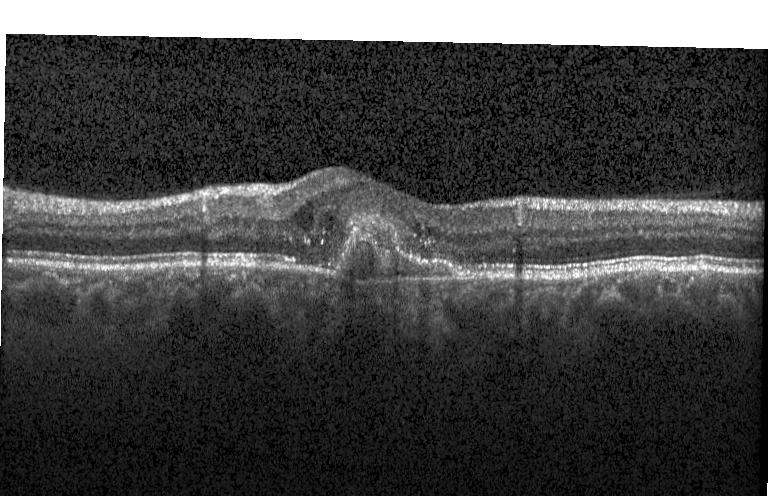 OCT B-scan.
OCT finding: CNV.